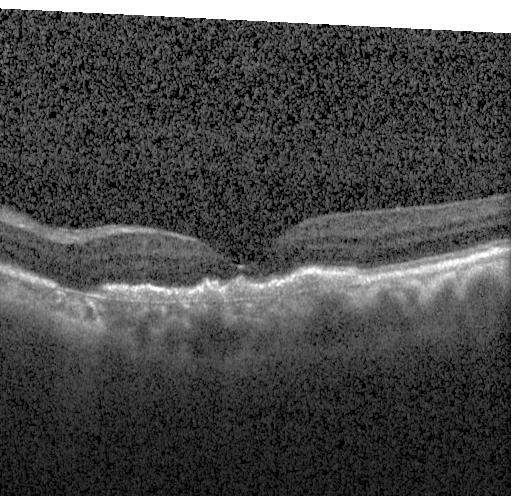 OCT B-scan; fovea-centered; spectral-domain optical coherence tomography; instrument: Heidelberg Spectralis.
Finding: CNV.